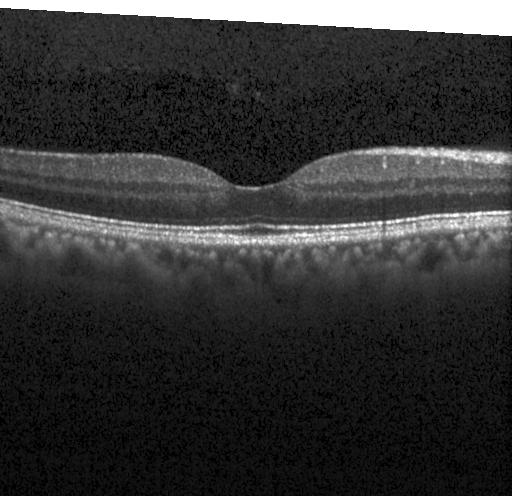

Retinal OCT cross-section.
Diagnosis: no CNV, DME, or drusen.